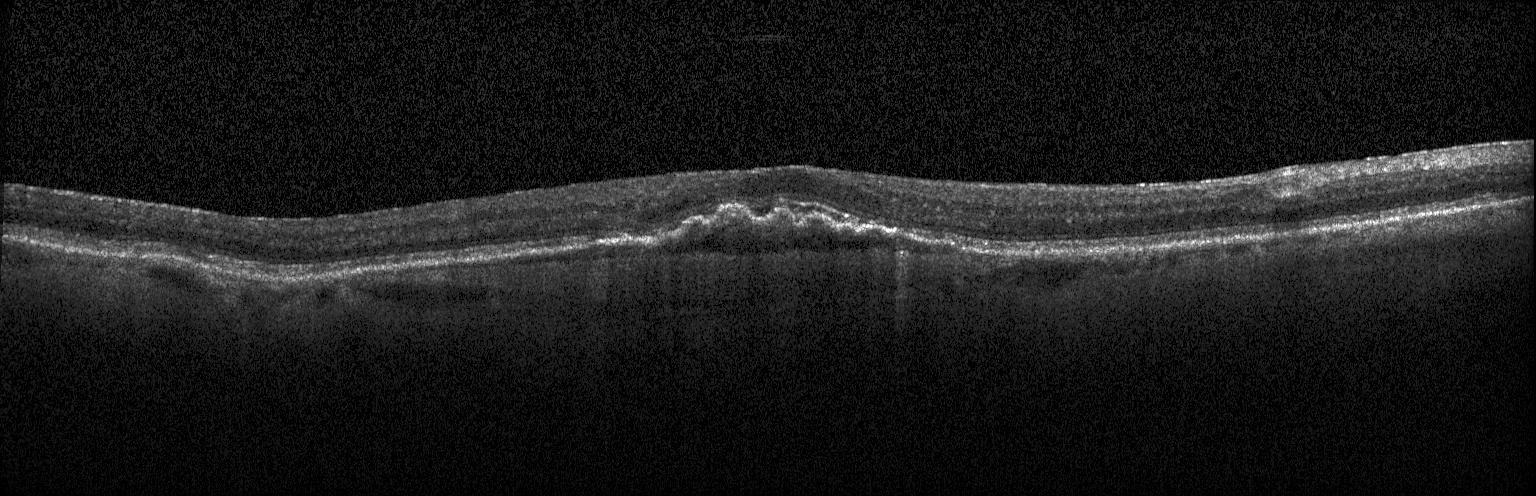 Macular OCT: a choroidal neovascular membrane.